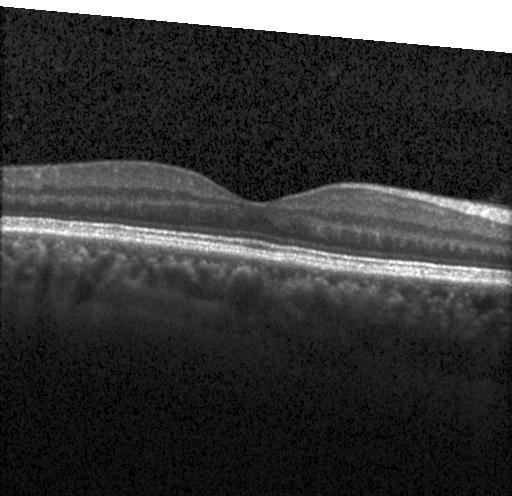 Retinal OCT cross-section; fovea-centered; acquired on a Heidelberg Spectralis. Assessment: no CNV, DME, or drusen.